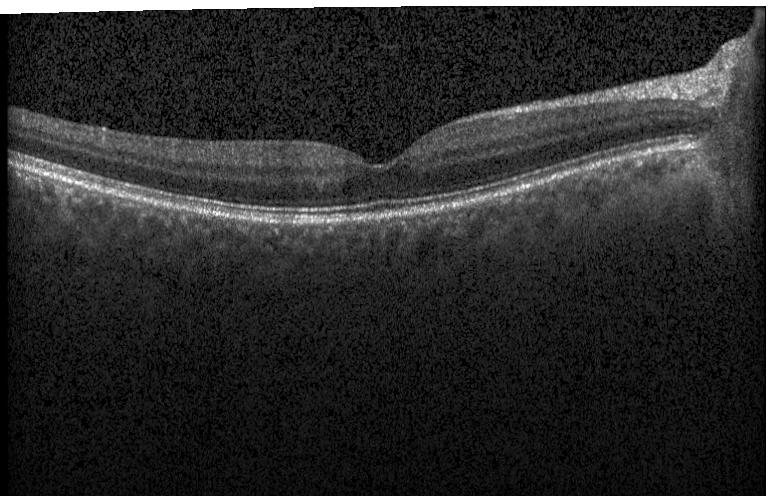

Macular scan, OCT B-scan, SD-OCT, acquired on a Heidelberg Spectralis.
The scan shows neither choroidal neovascularization, diabetic macular edema, nor drusen.